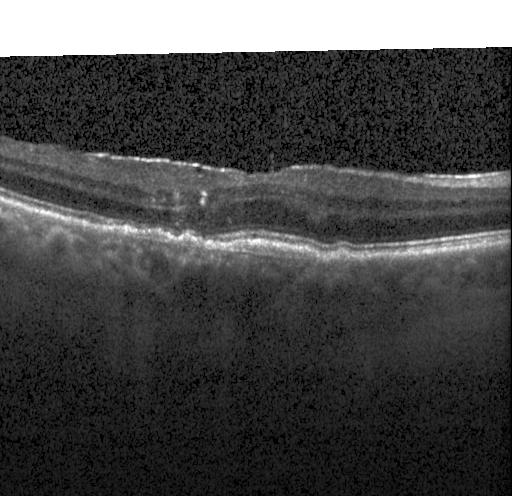
Retinal OCT cross-section
Dx: choroidal neovascularization.